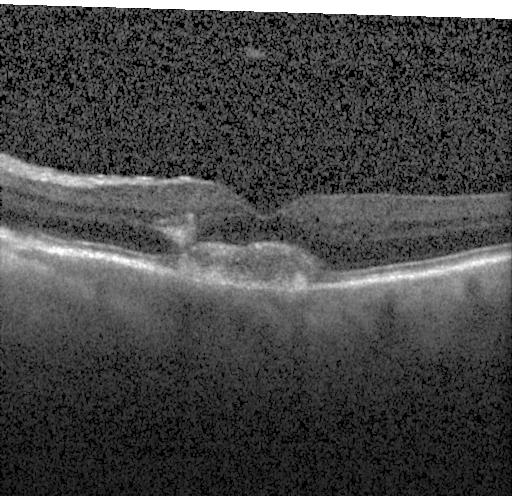 OCT line scan
Finding: CNV.